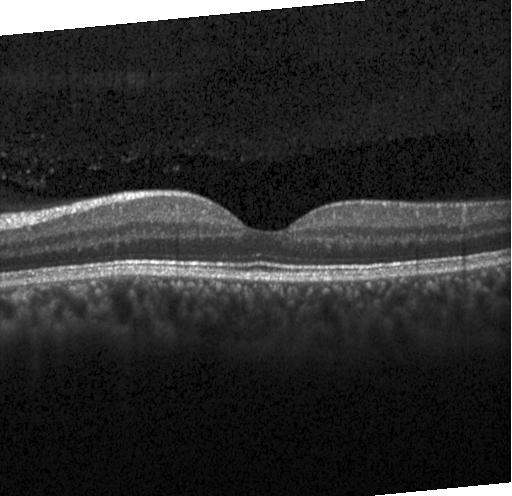 Through the macula. Optical coherence tomography B-scan. Spectral-domain OCT. Instrument: Heidelberg Spectralis
No choroidal neovascularization, no diabetic macular edema, and no drusen.